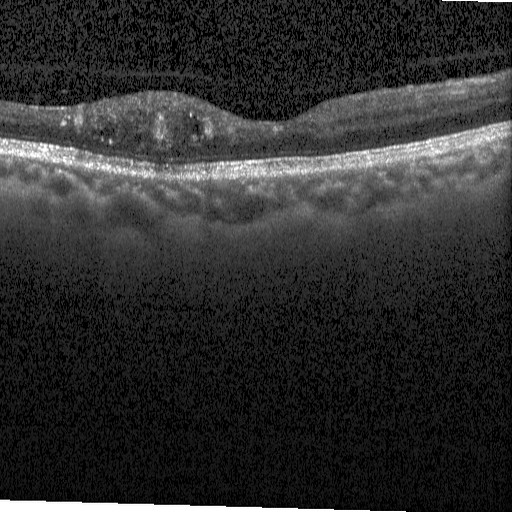
OCT B-scan.
Diagnosis: diabetic macular edema (DME).